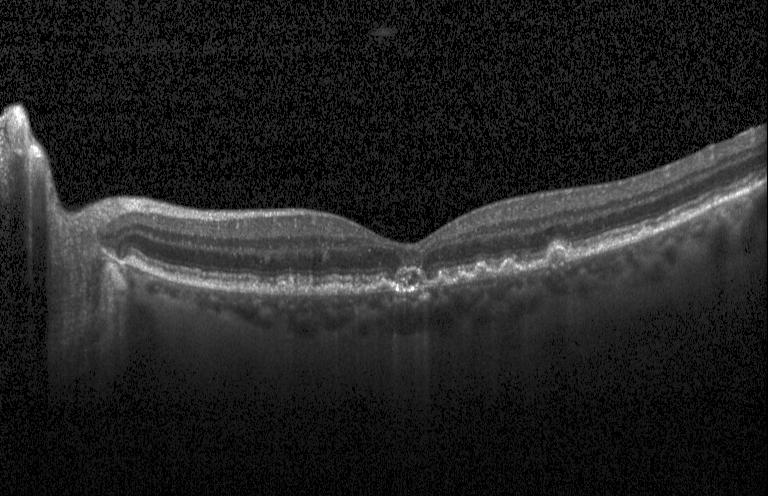

Retinal OCT B-scan; Heidelberg Spectralis OCT system; SD-OCT; horizontal scan through the fovea — Finding: a choroidal neovascular membrane.